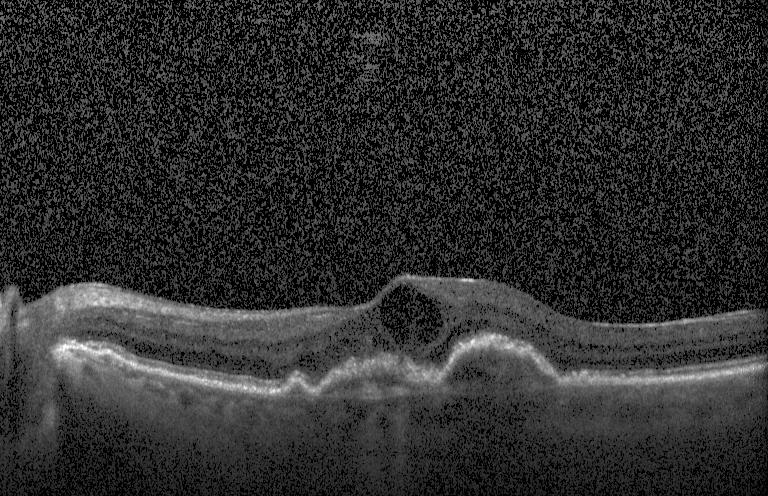 Optical coherence tomography B-scan. Choroidal neovascularization.